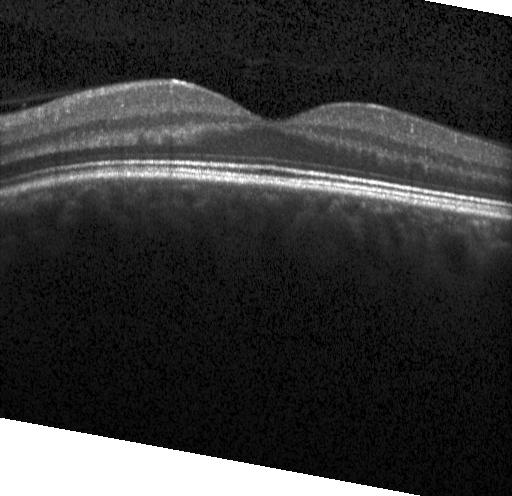

Through the macula · spectral-domain optical coherence tomography · Heidelberg Spectralis OCT system · OCT line scan — Finding: neither CNV, DME, nor drusen.